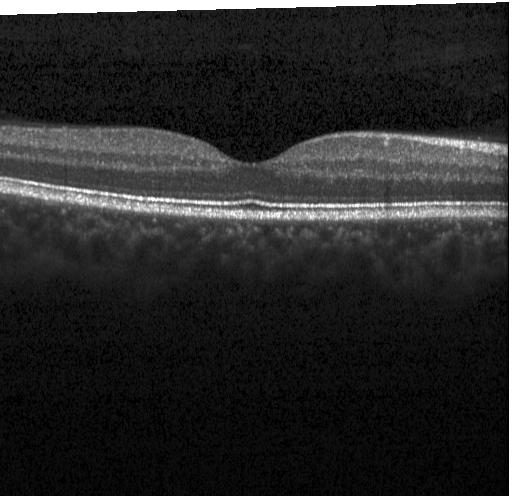
Spectral-domain OCT B-scan: no choroidal neovascularization, no diabetic macular edema, and no drusen.